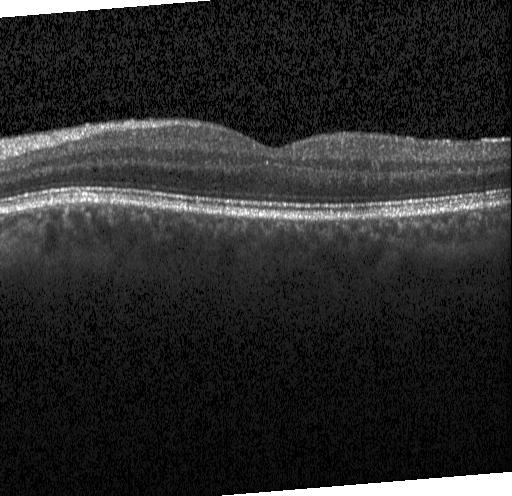
Through the macula, SD-OCT, optical coherence tomography scan, acquired on a Heidelberg Spectralis — The scan shows no evidence of choroidal neovascularization, diabetic macular edema, or drusen.